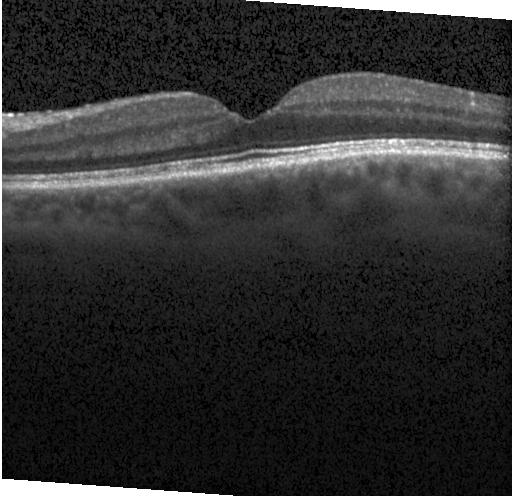
Through the macula. Spectral-domain optical coherence tomography. Heidelberg Spectralis OCT system. OCT line scan
Finding: neither CNV, DME, nor drusen.